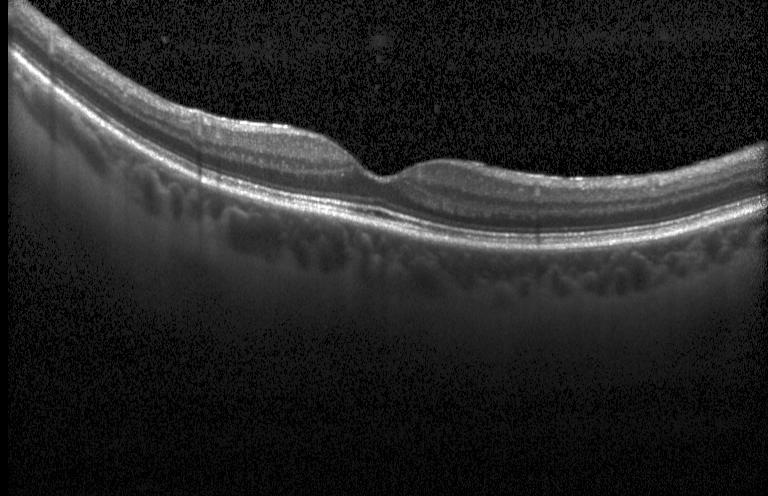 Spectral-domain optical coherence tomography. Optical coherence tomography B-scan — Diagnosis: no evidence of CNV, DME, or drusen.